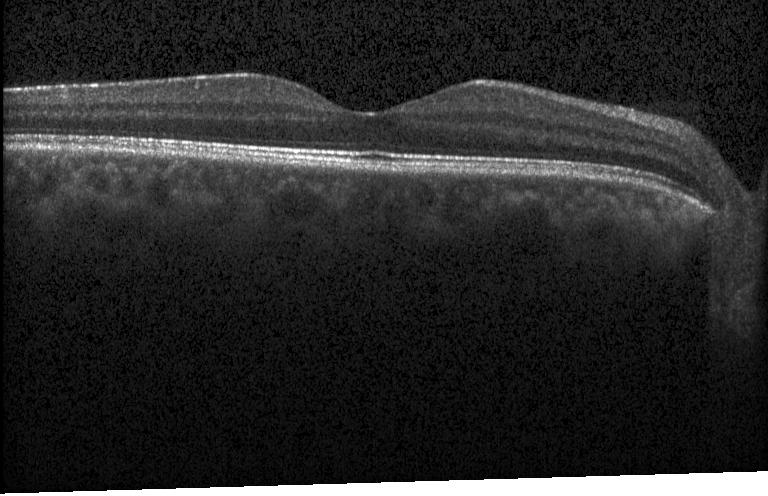 Optical coherence tomography scan — Diagnosis: no evidence of CNV, DME, or drusen.